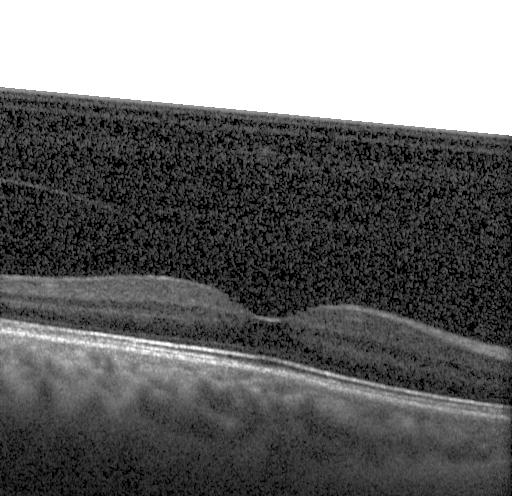 Fovea-centered · instrument: Heidelberg Spectralis · OCT B-scan. This B-scan demonstrates no CNV, no DME, and no drusen.